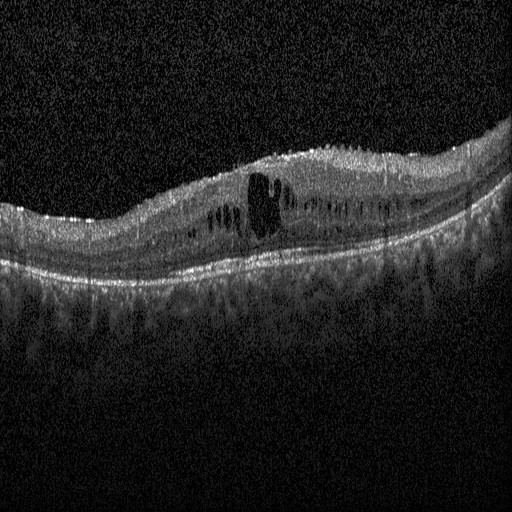 Retinal OCT cross-section
This B-scan demonstrates diabetic macular edema.